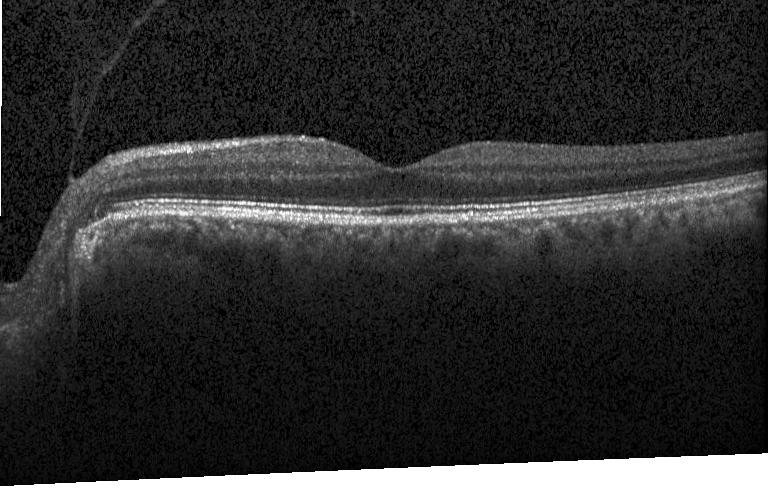

OCT finding: no CNV, no DME, and no drusen.